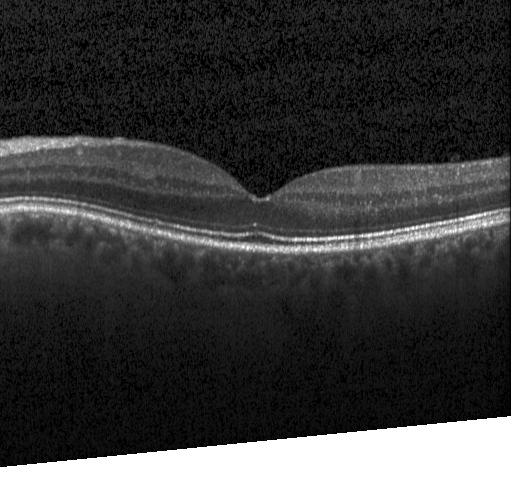
Impression: no CNV, no DME, and no drusen.